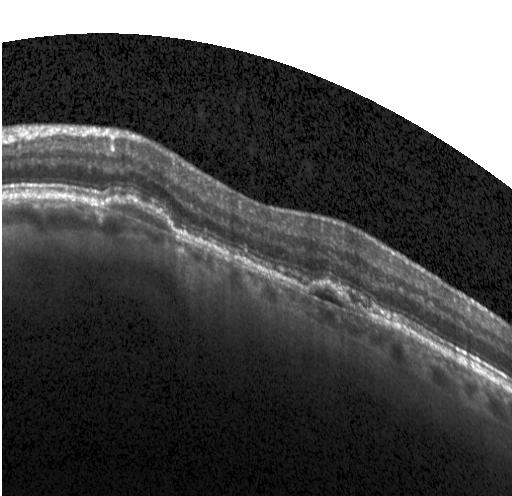

OCT line scan.
OCT finding: a choroidal neovascular membrane.